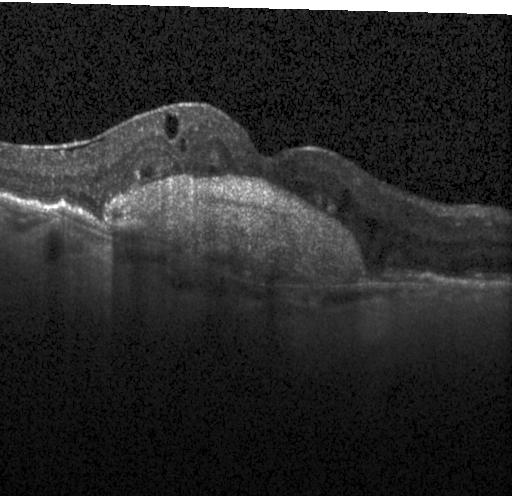 Impression: a choroidal neovascular membrane.